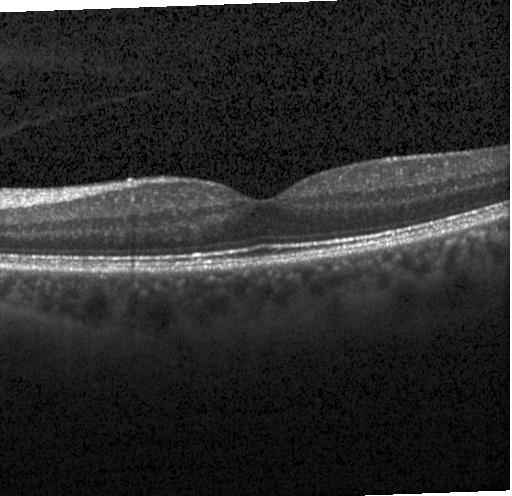

Optical coherence tomography scan. Fovea-centered
Diagnosis: no evidence of choroidal neovascularization, diabetic macular edema, or drusen.